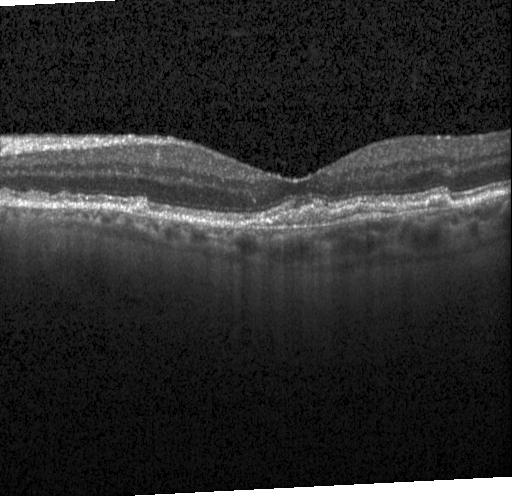
Diagnosis: a choroidal neovascular membrane.